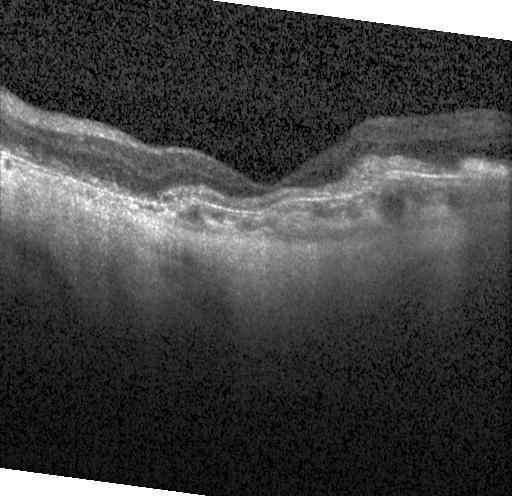 Retinal OCT cross-section. SD-OCT
Diagnosis: CNV.